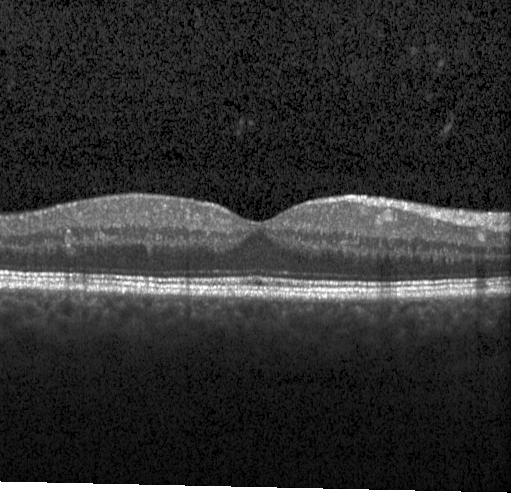

Spectral-domain optical coherence tomography · optical coherence tomography B-scan. Dx: no CNV, DME, or drusen.